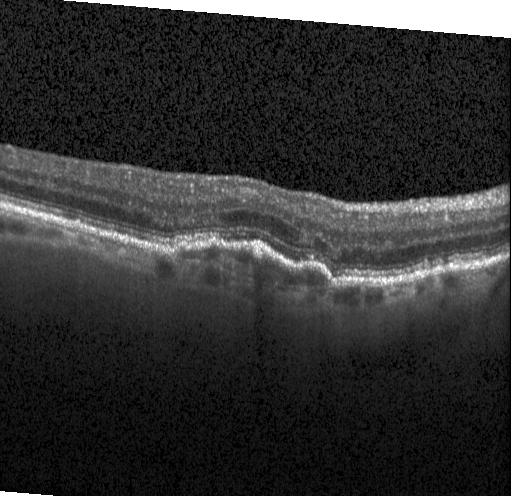 Retinal OCT cross-section · SD-OCT
The scan shows choroidal neovascularization.